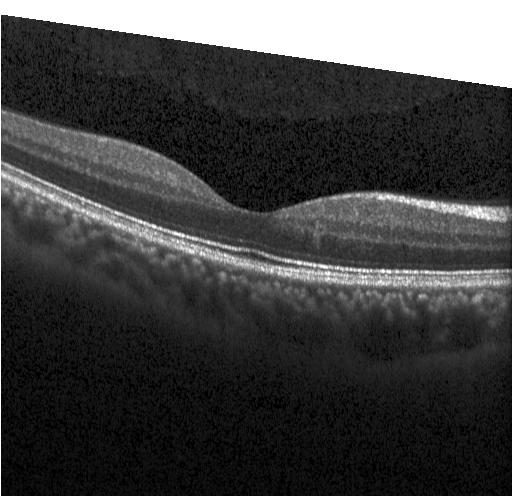

Spectral-domain optical coherence tomography. Retinal OCT cross-section. Through the macula. Diagnosis: no evidence of choroidal neovascularization, diabetic macular edema, or drusen.